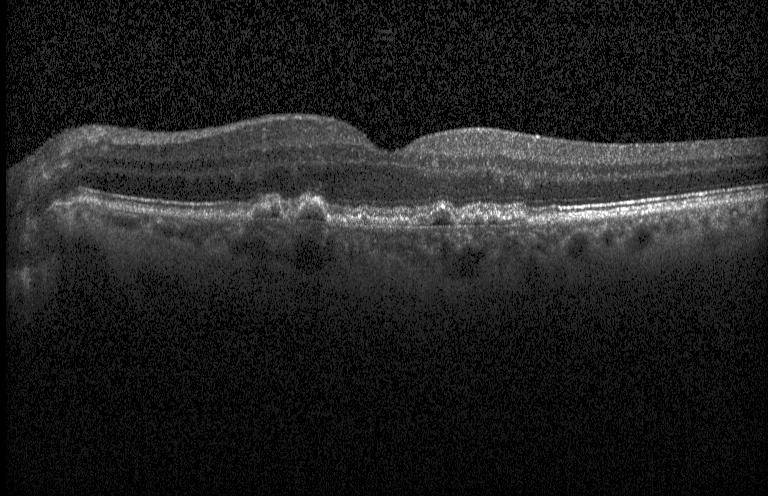
Retinal OCT B-scan. Impression: sub-RPE drusenoid deposits.